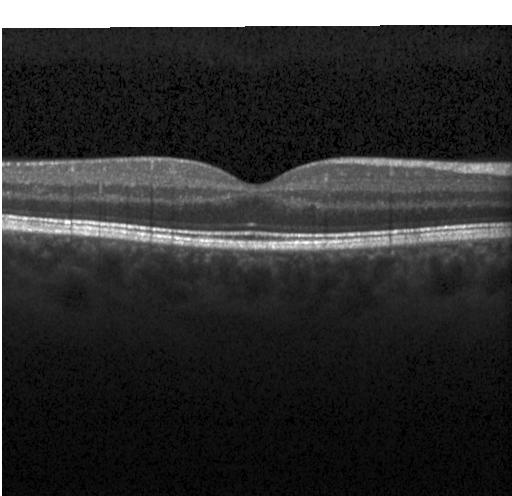

Spectral-domain optical coherence tomography. Retinal OCT cross-section. Heidelberg Spectralis OCT system. Macular OCT: no CNV, DME, or drusen.